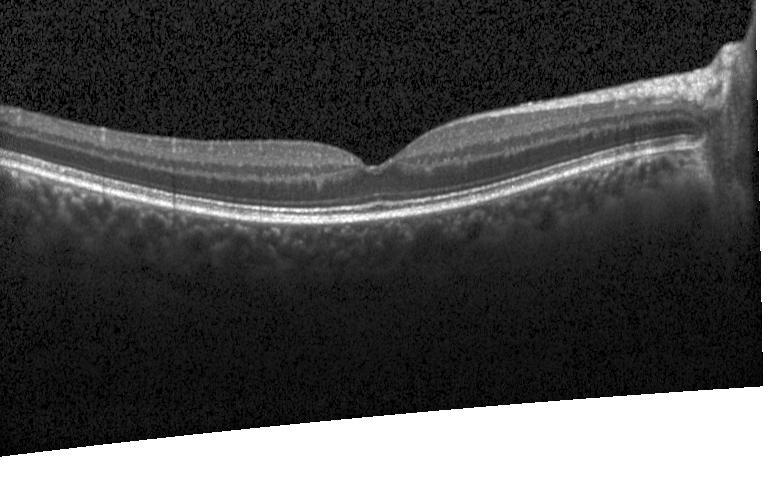 The scan shows no evidence of choroidal neovascularization, diabetic macular edema, or drusen.